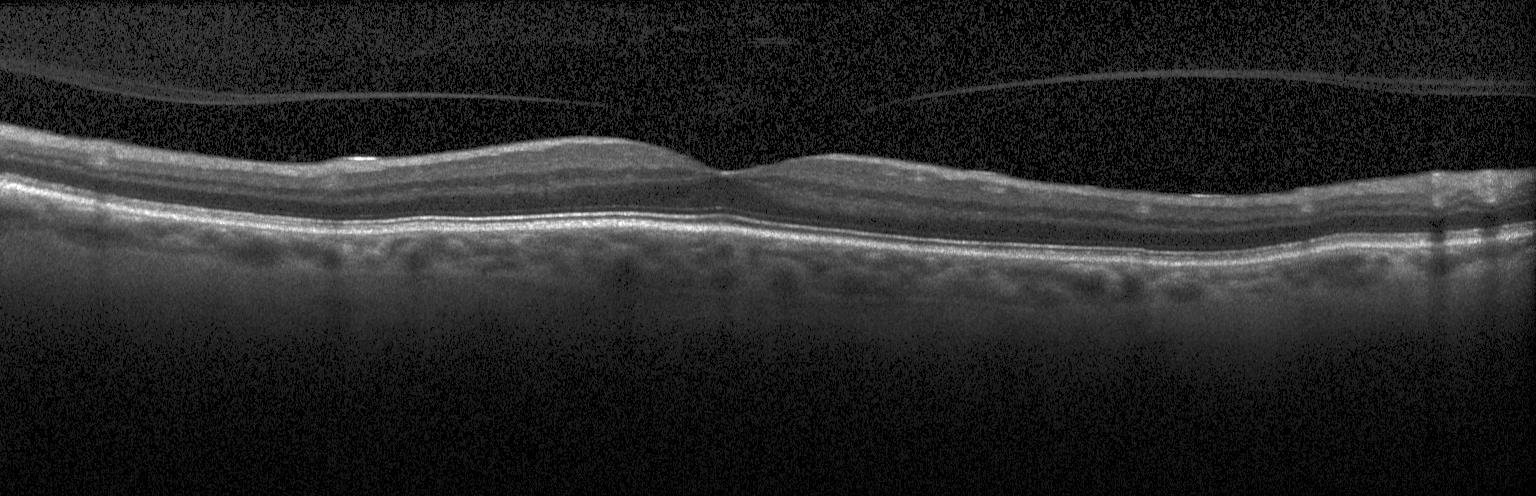 This B-scan demonstrates no evidence of choroidal neovascularization, diabetic macular edema, or drusen.